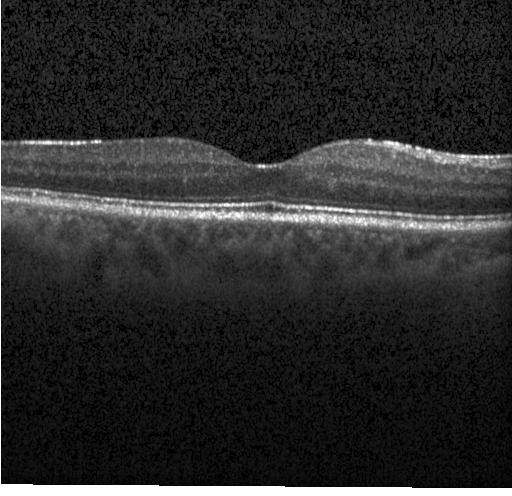
Fovea-centered · optical coherence tomography B-scan.
No choroidal neovascularization, diabetic macular edema, or drusen.